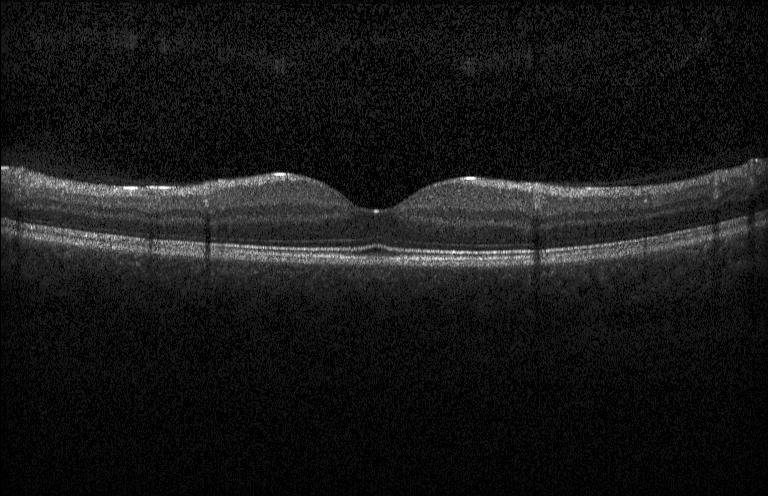 Spectral-domain optical coherence tomography. OCT B-scan — Neither CNV, DME, nor drusen.